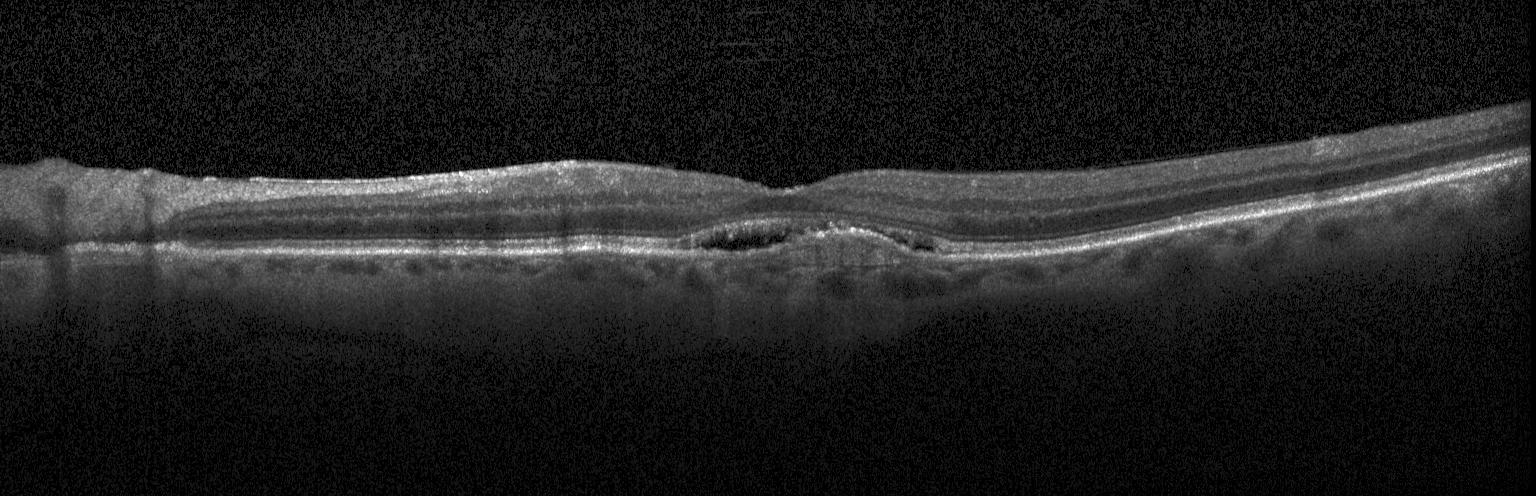

Spectral-domain optical coherence tomography; optical coherence tomography B-scan; horizontal scan through the fovea; acquired on a Heidelberg Spectralis
Diagnosis: a choroidal neovascular membrane.